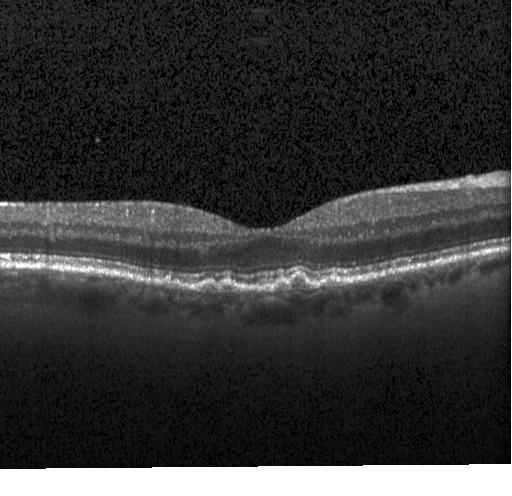 This B-scan demonstrates drusen.